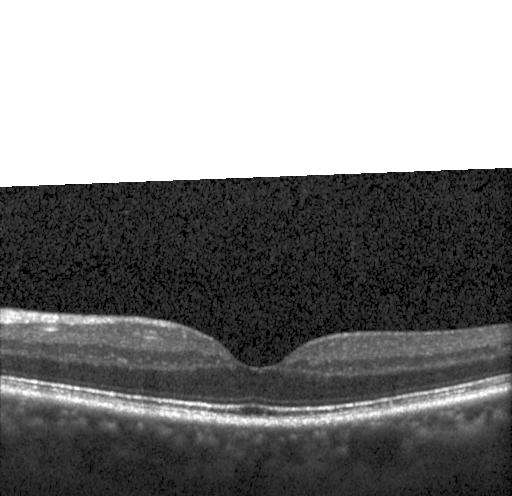

Optical coherence tomography scan
Finding: no choroidal neovascularization, diabetic macular edema, or drusen.